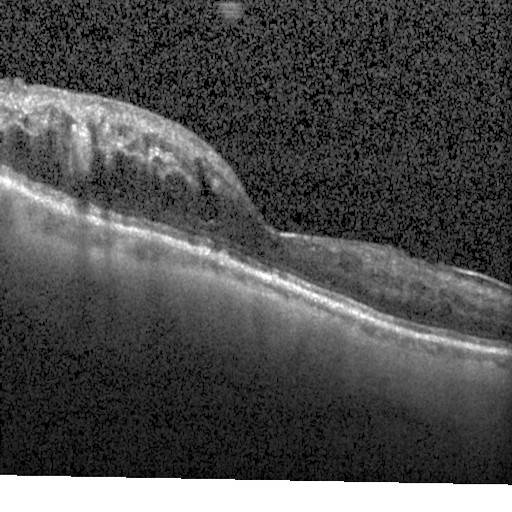 Heidelberg Spectralis OCT system; OCT B-scan; horizontal scan through the fovea; SD-OCT
Diabetic macular edema (DME).